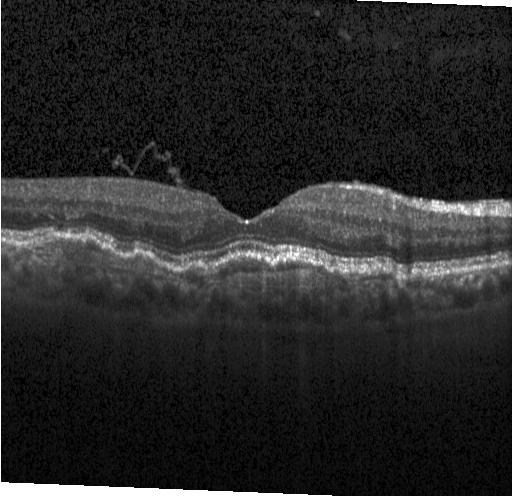

Macular scan · retinal OCT B-scan · instrument: Heidelberg Spectralis — Finding: a choroidal neovascular membrane.